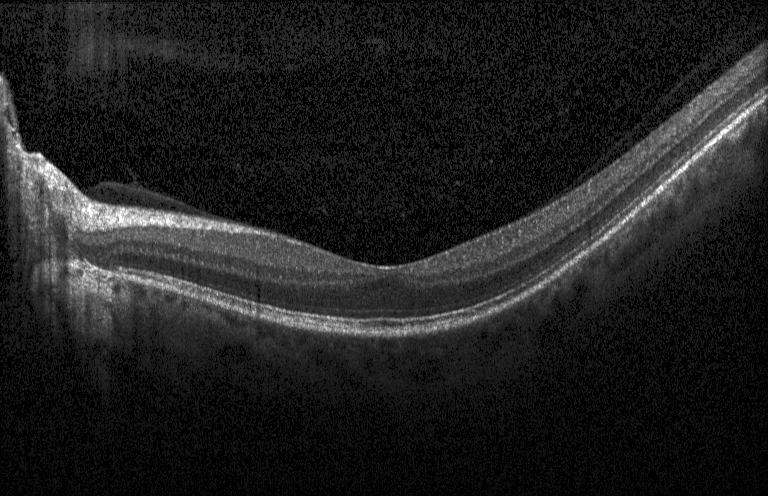

Impression: no evidence of CNV, DME, or drusen.